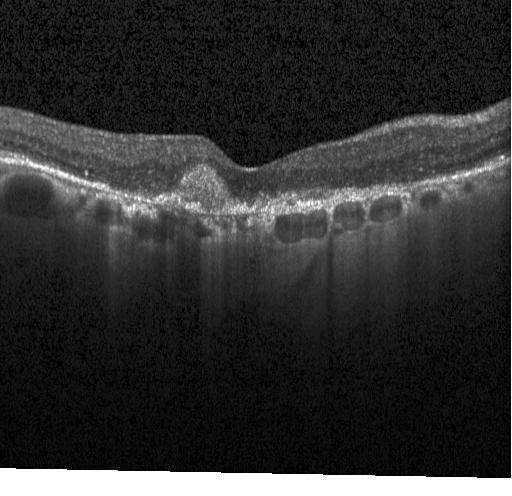

Diagnosis: a choroidal neovascular membrane.